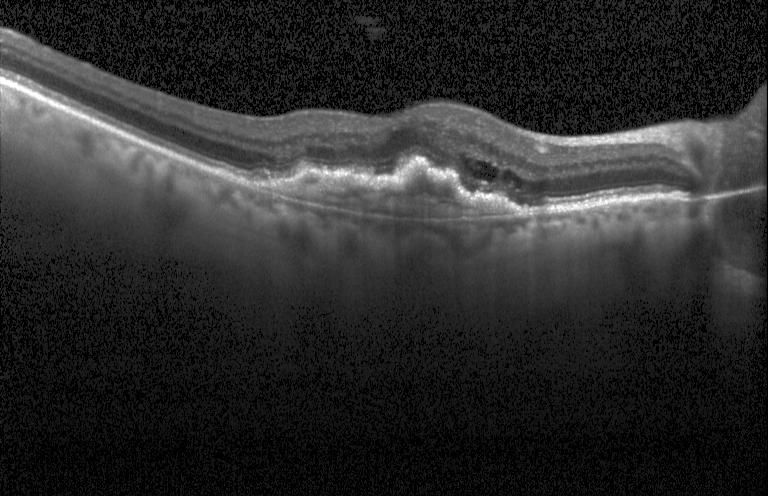 Retinal OCT B-scan — Assessment: choroidal neovascularization.